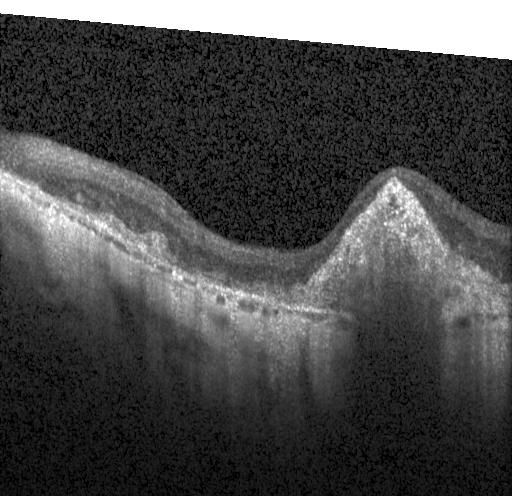

Retinal OCT B-scan. OCT finding: choroidal neovascularization.